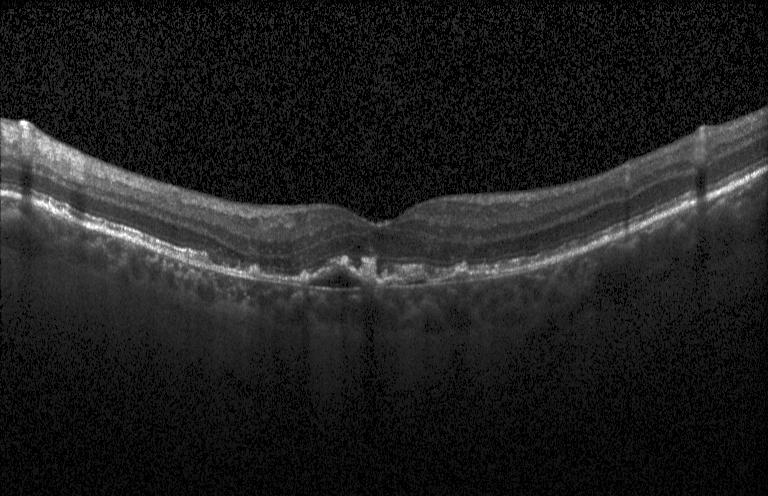
Fovea-centered. Optical coherence tomography scan. Spectral-domain optical coherence tomography. Acquired on a Heidelberg Spectralis
Finding: CNV.